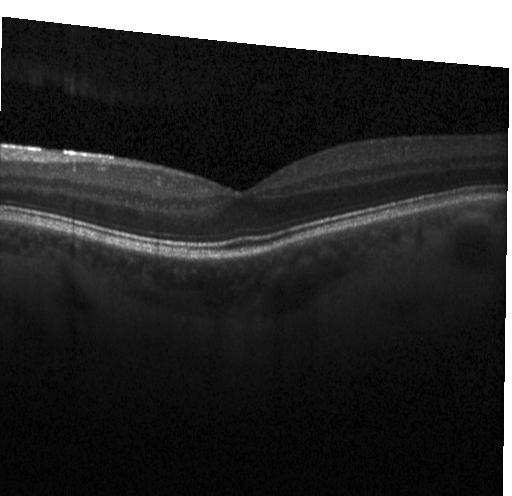
Centered on the fovea. Acquired on a Heidelberg Spectralis. Spectral-domain optical coherence tomography. Optical coherence tomography scan. The scan shows no evidence of CNV, DME, or drusen.